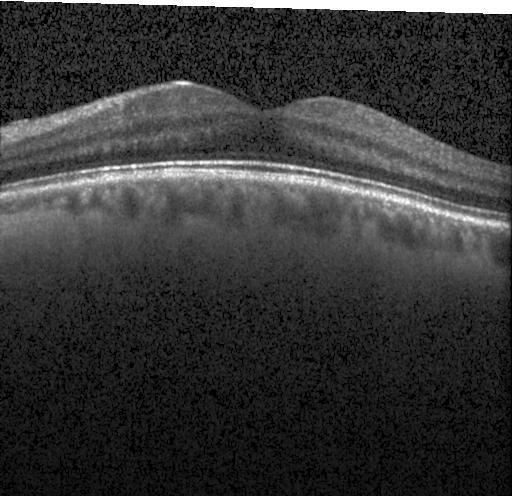

Impression: no evidence of choroidal neovascularization, diabetic macular edema, or drusen.